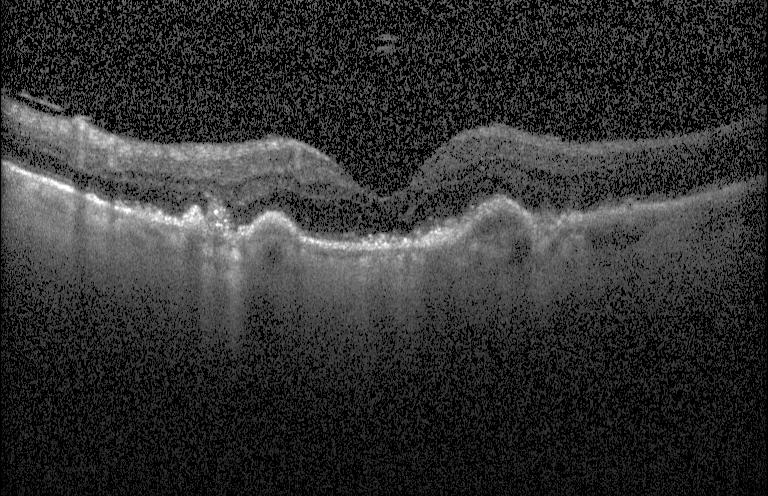
Finding: CNV.